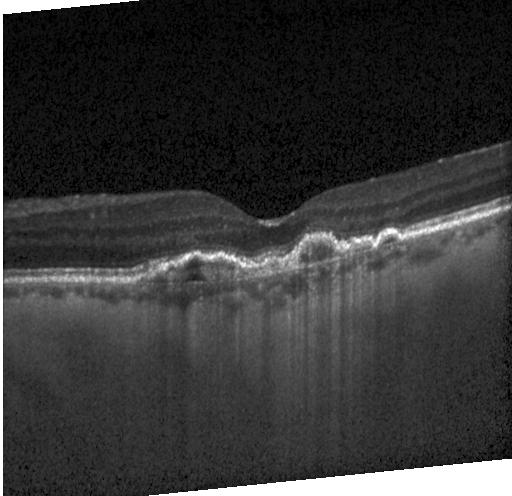

OCT B-scan.
Dx: a choroidal neovascular membrane.